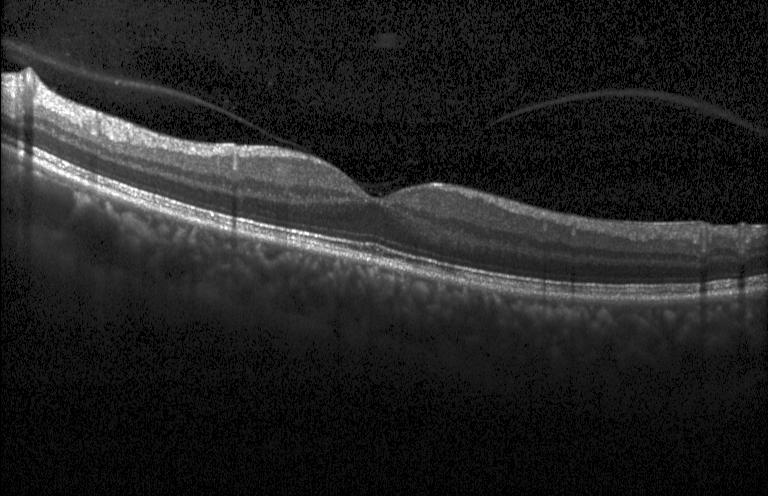

Optical coherence tomography scan. Assessment: no CNV, DME, or drusen.